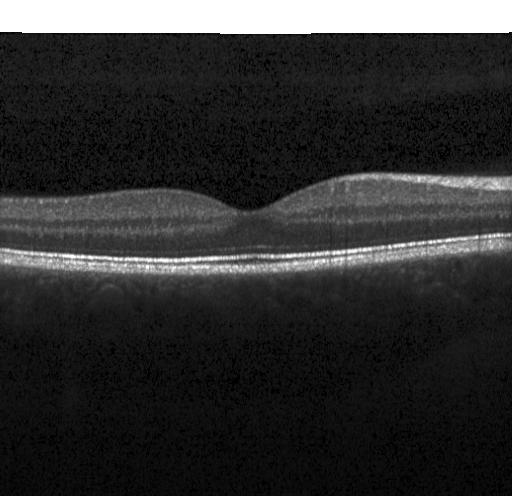
OCT B-scan — Assessment: no evidence of CNV, DME, or drusen.